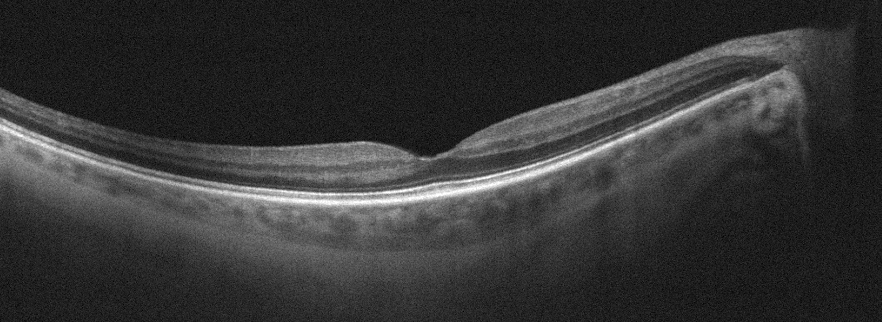 This B-scan demonstrates age-related macular degeneration (AMD).